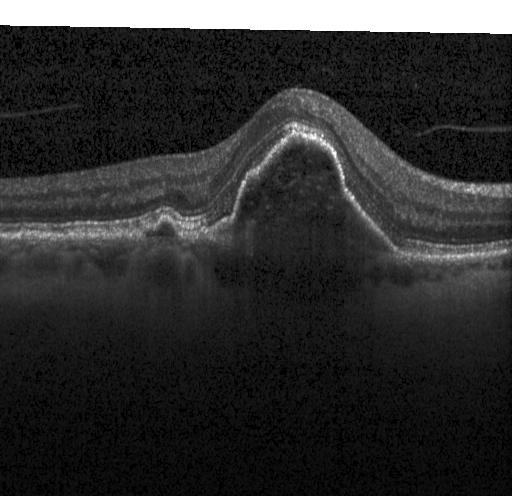

This B-scan demonstrates CNV.